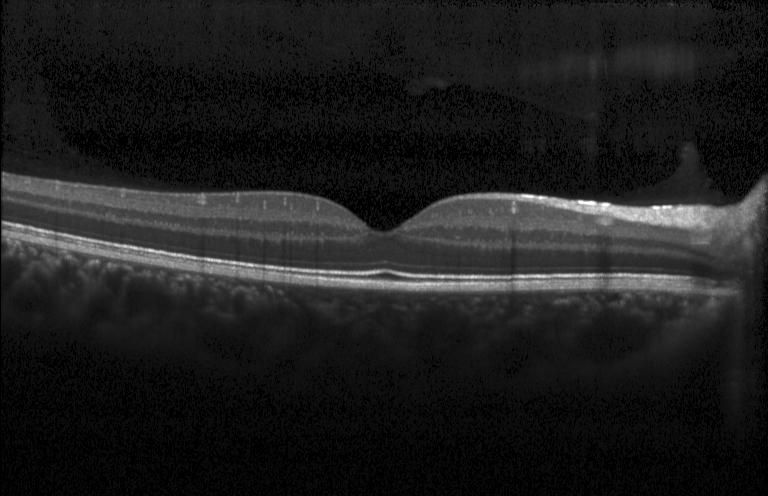 Optical coherence tomography scan — Finding: no CNV, no DME, and no drusen.